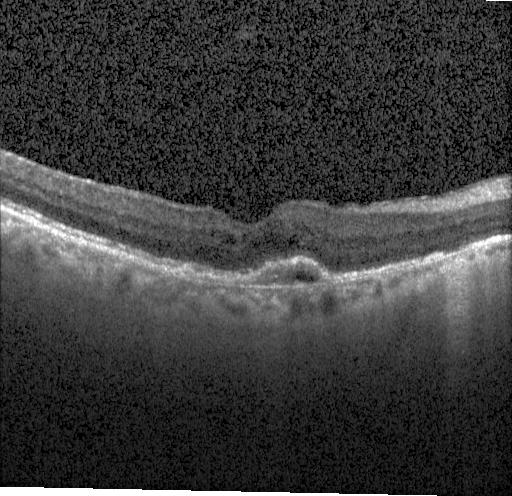
Spectral-domain optical coherence tomography. Horizontal scan through the fovea. Optical coherence tomography scan. Instrument: Heidelberg Spectralis — Dx: CNV.